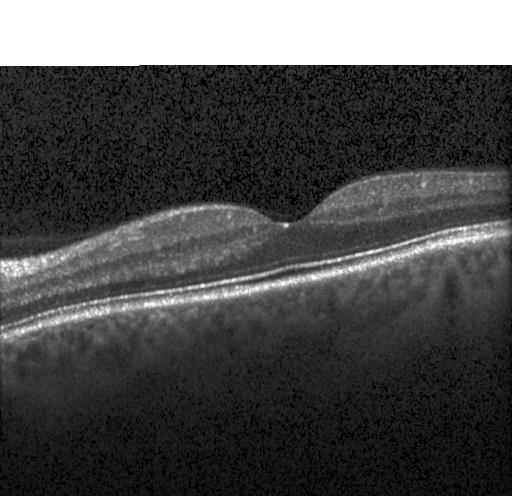
Optical coherence tomography B-scan
Diagnosis: no choroidal neovascularization, no diabetic macular edema, and no drusen.